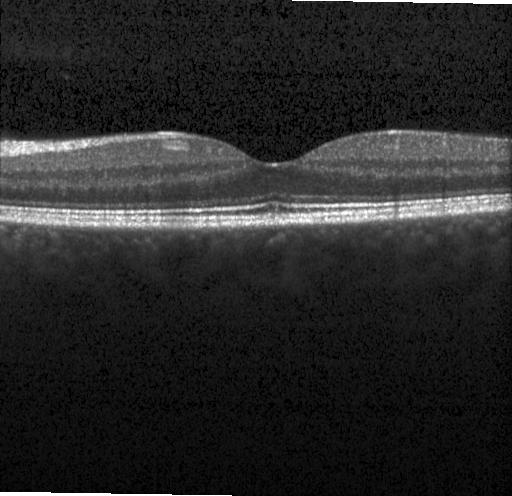 Acquired on a Heidelberg Spectralis, optical coherence tomography scan.
Finding: neither CNV, DME, nor drusen.